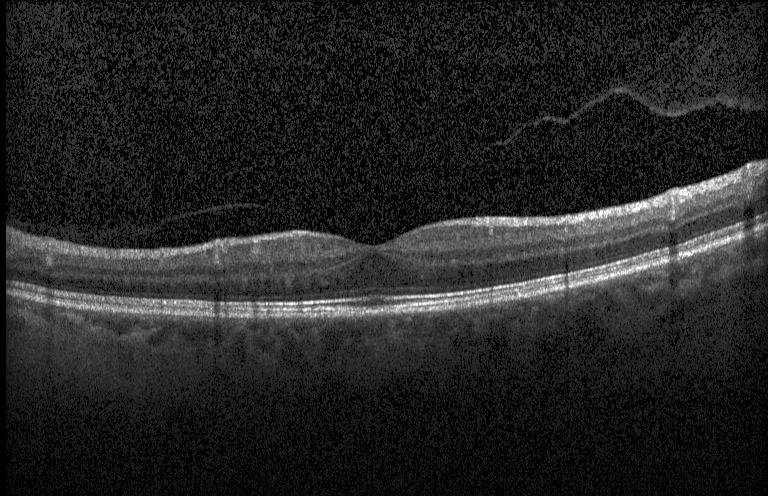

Macular OCT: no CNV, no DME, and no drusen.